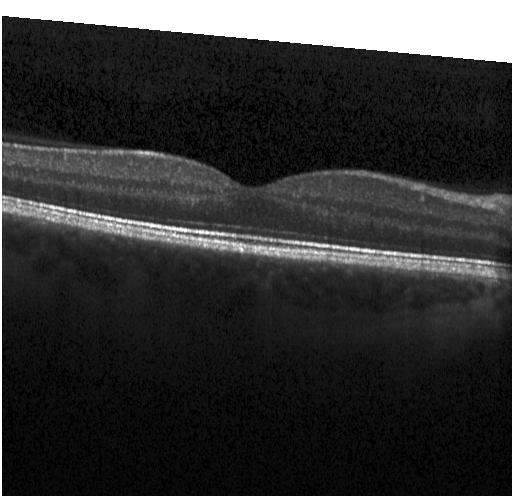
No choroidal neovascularization, no diabetic macular edema, and no drusen.